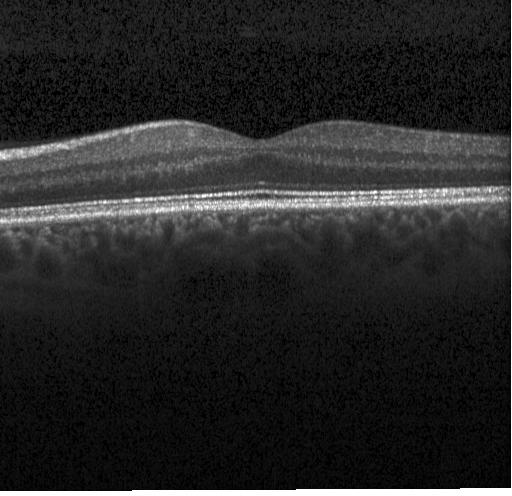 Retinal OCT cross-section showing no choroidal neovascularization, no diabetic macular edema, and no drusen.